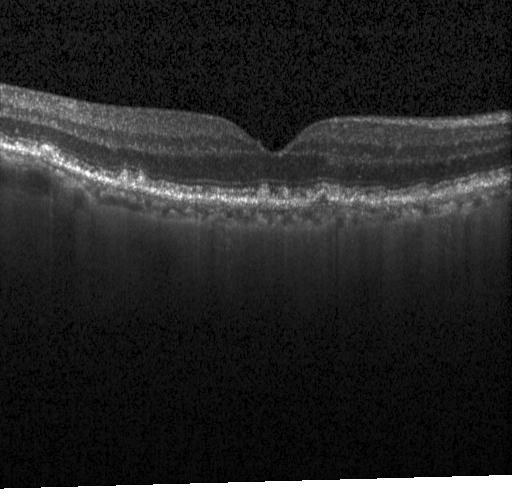
Retinal OCT cross-section showing sub-RPE drusenoid deposits.